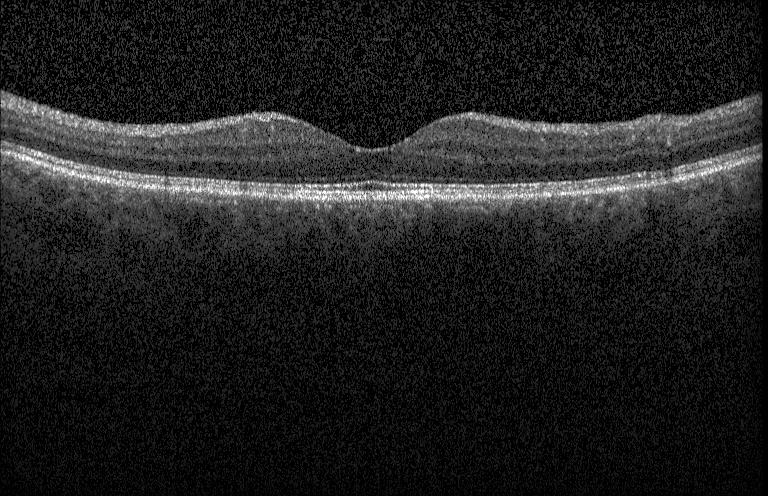
This B-scan demonstrates neither CNV, DME, nor drusen.